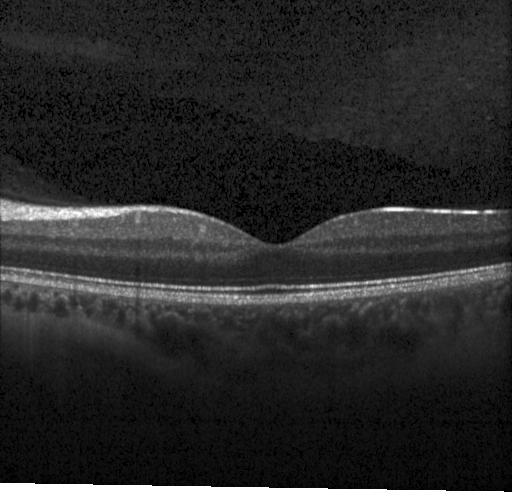

OCT line scan. SD-OCT. Centered on the fovea — OCT finding: neither CNV, DME, nor drusen.